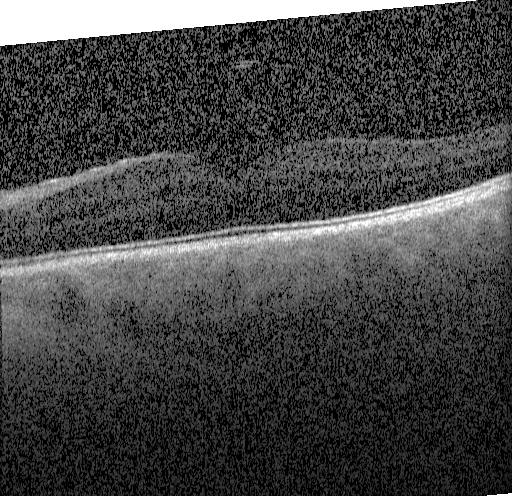 This B-scan demonstrates no choroidal neovascularization, no diabetic macular edema, and no drusen.